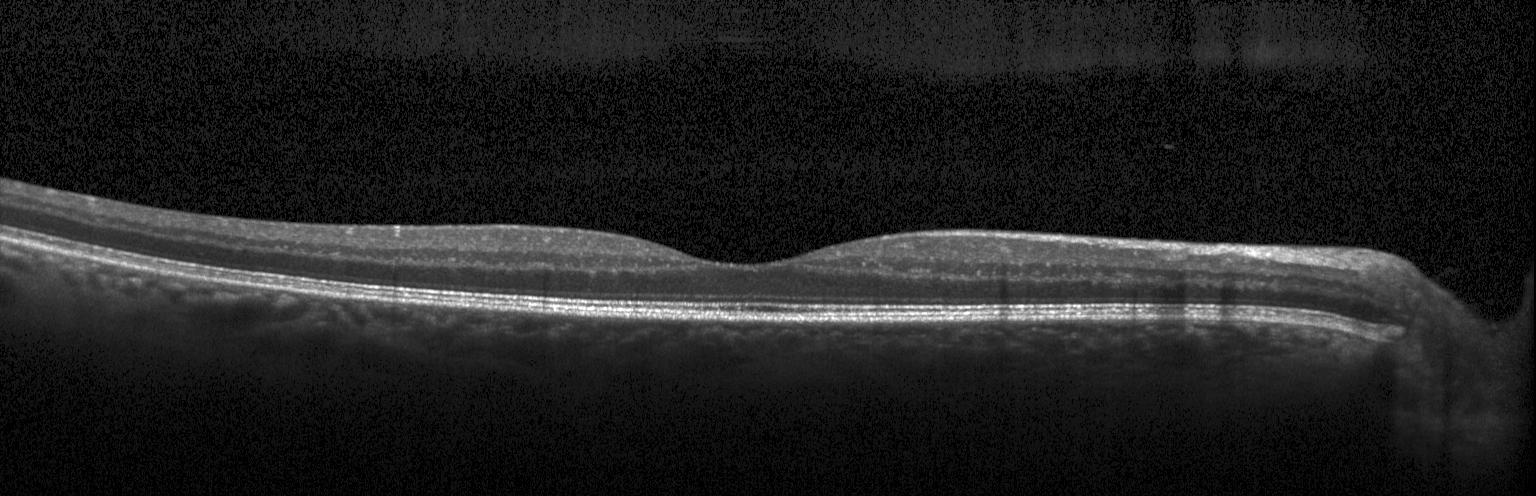

OCT B-scan.
Dx: neither choroidal neovascularization, diabetic macular edema, nor drusen.